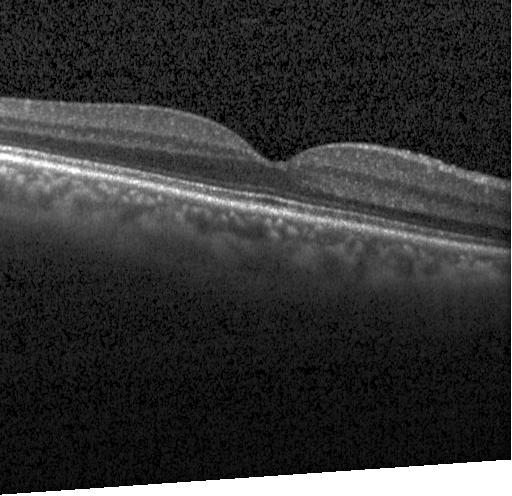 Through the macula; optical coherence tomography scan; spectral-domain OCT.
Dx: no choroidal neovascularization, no diabetic macular edema, and no drusen.